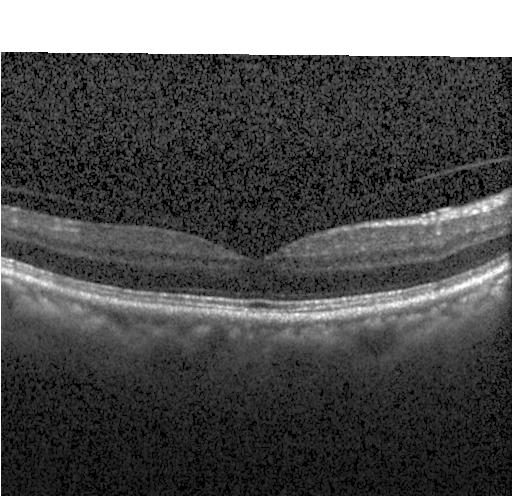

OCT B-scan showing neither choroidal neovascularization, diabetic macular edema, nor drusen.